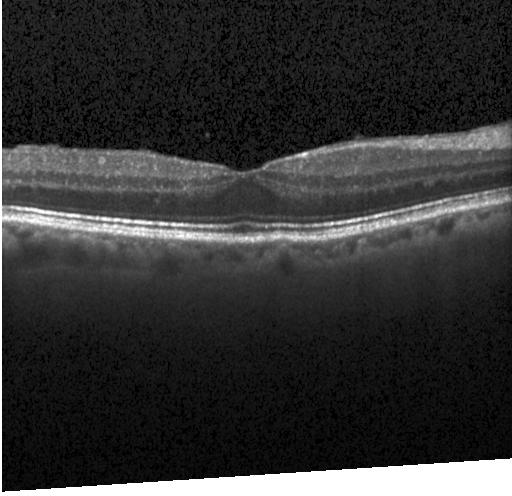

SD-OCT. Centered on the fovea. OCT B-scan — No choroidal neovascularization, no diabetic macular edema, and no drusen.